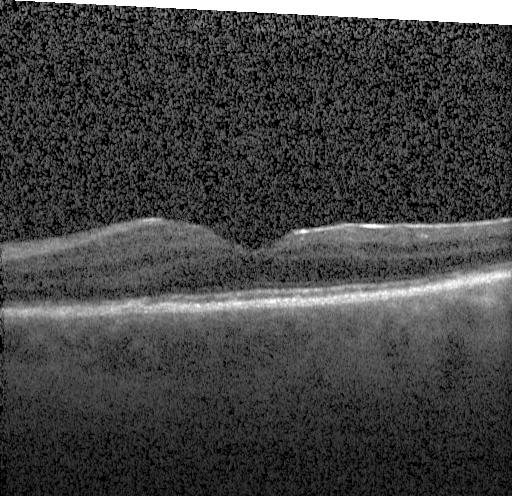
Centered on the fovea, optical coherence tomography scan — Impression: no choroidal neovascularization, diabetic macular edema, or drusen.